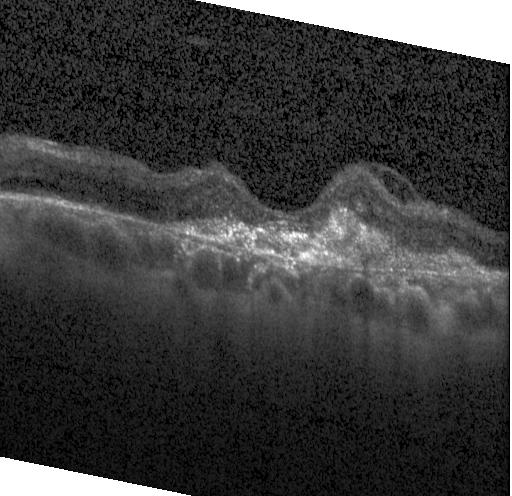 Heidelberg Spectralis OCT system; spectral-domain OCT; fovea-centered; retinal OCT cross-section. Assessment: CNV.